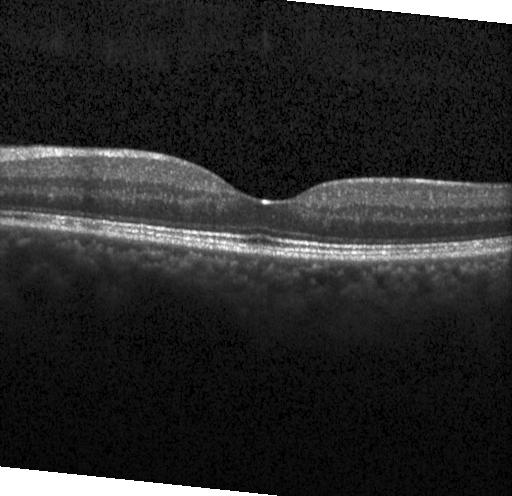 Finding: no evidence of CNV, DME, or drusen.